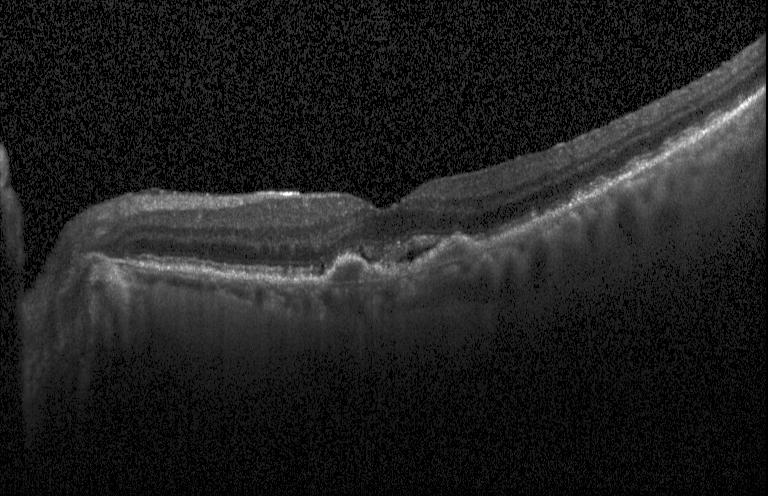

Macular OCT demonstrating a choroidal neovascular membrane.